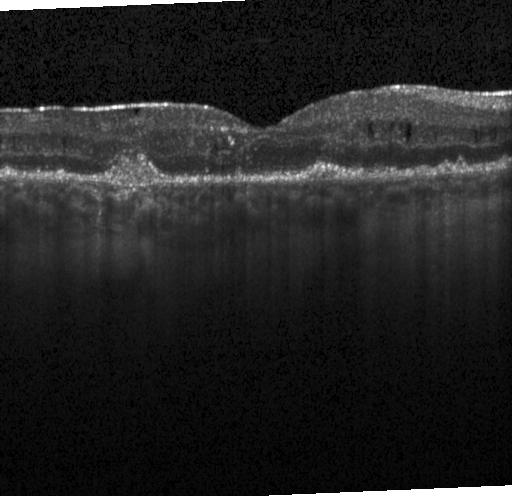

Through the macula · optical coherence tomography B-scan · Heidelberg Spectralis · SD-OCT.
The scan shows a choroidal neovascular membrane.